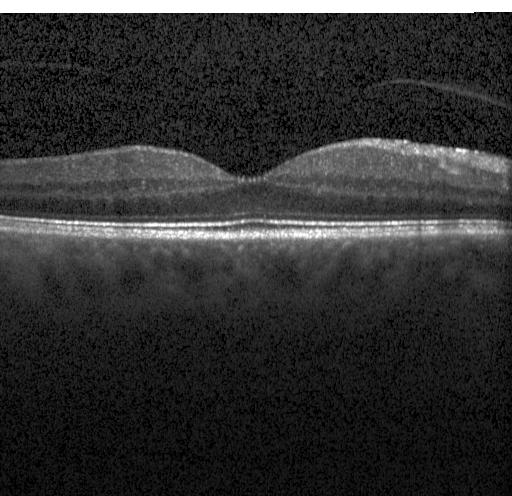 Impression: no CNV, no DME, and no drusen.